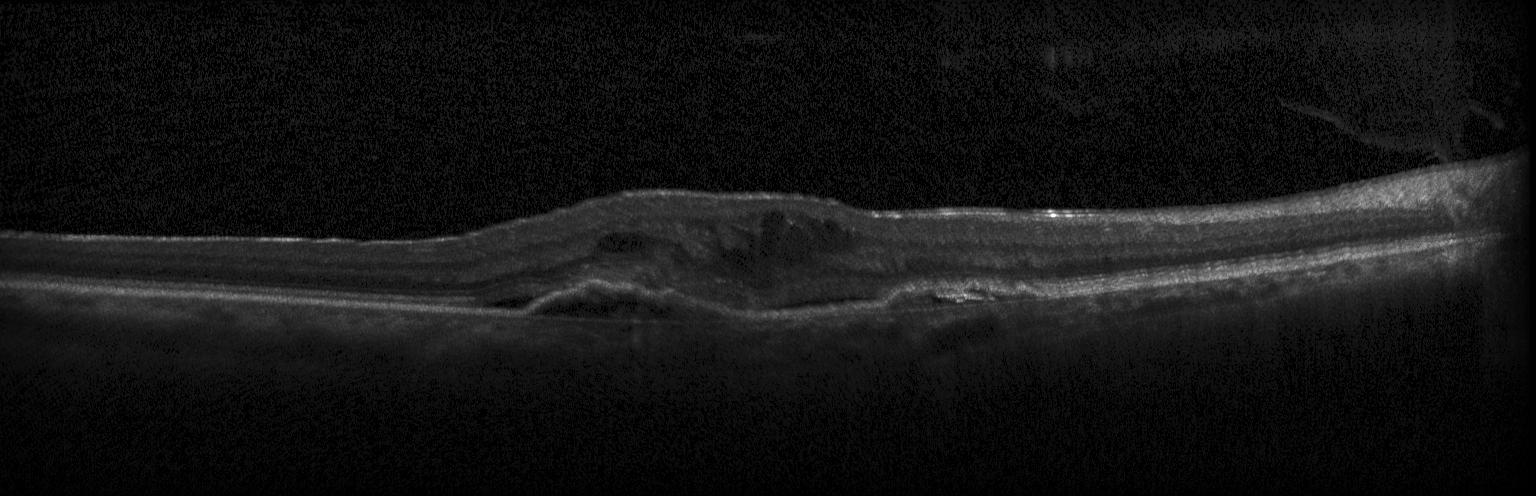

Macular scan · optical coherence tomography scan · spectral-domain optical coherence tomography · Heidelberg Spectralis.
Dx: CNV.